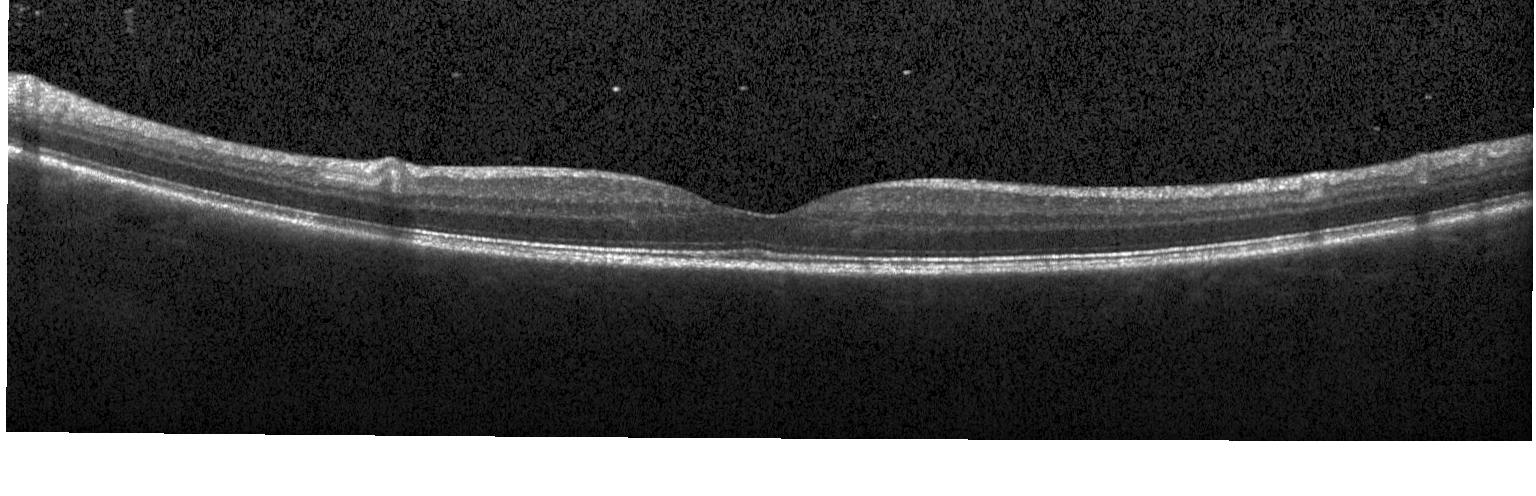

Heidelberg Spectralis; optical coherence tomography scan; horizontal scan through the fovea. No CNV, DME, or drusen.